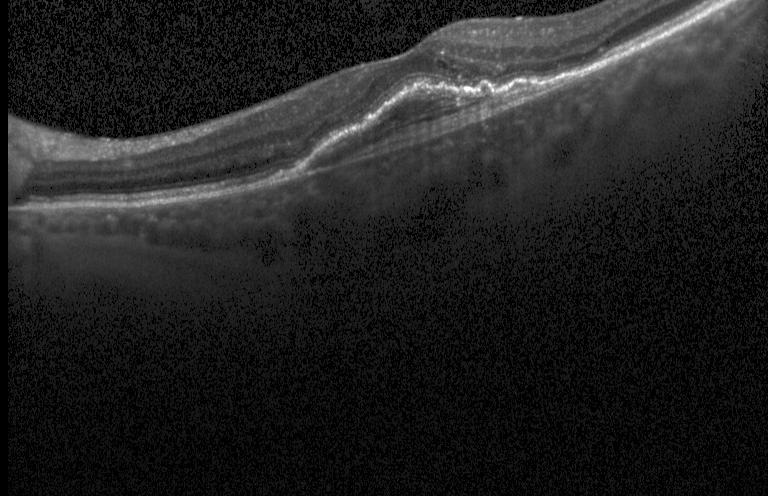
Finding: a choroidal neovascular membrane.